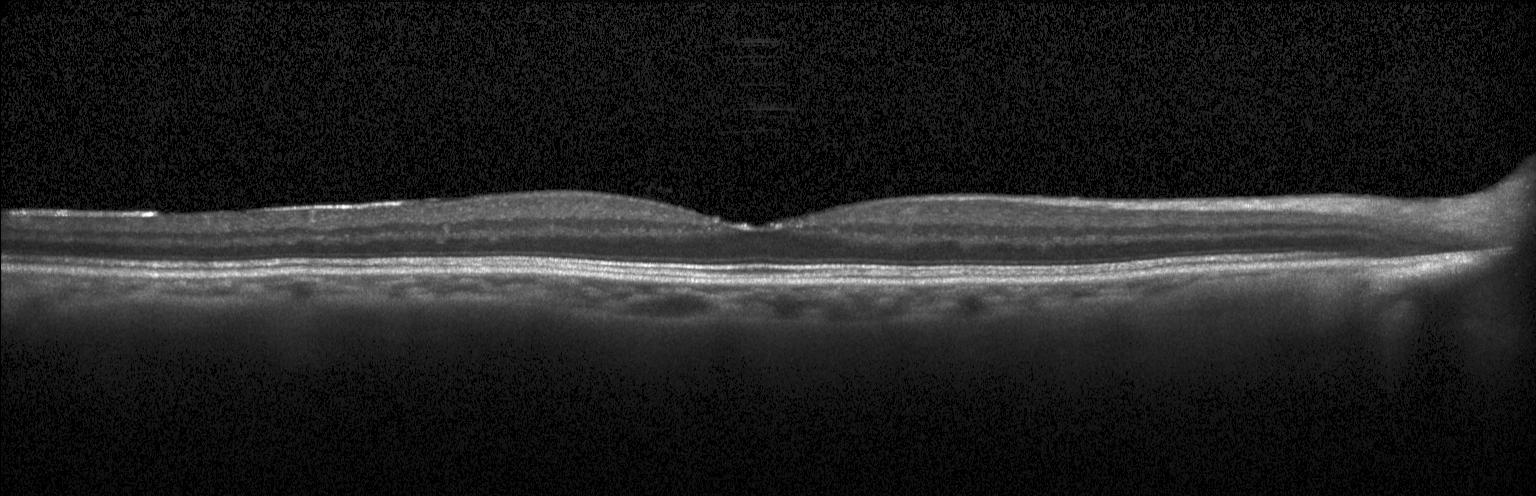 Macular OCT demonstrating neither CNV, DME, nor drusen.